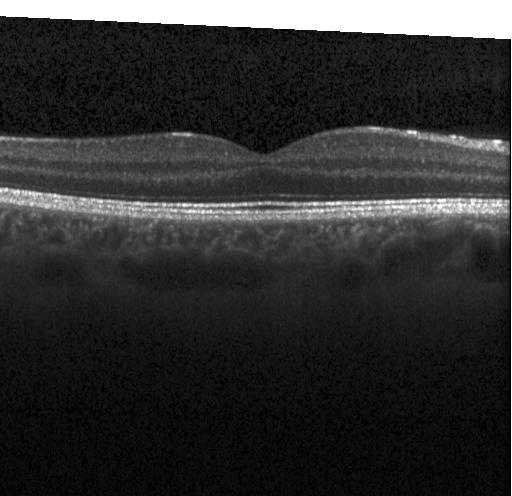
Acquired on a Heidelberg Spectralis, optical coherence tomography B-scan, fovea-centered
No choroidal neovascularization, diabetic macular edema, or drusen.